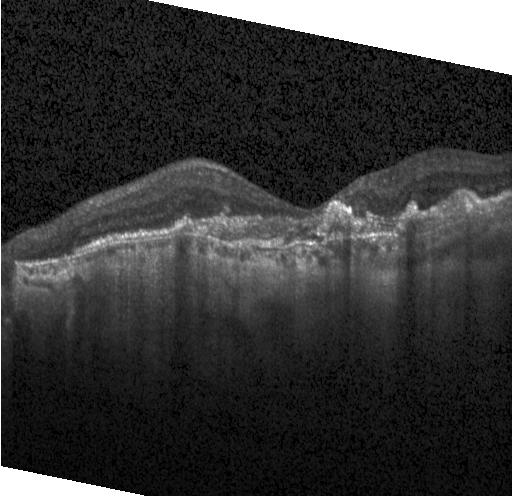 Retinal OCT cross-section; macular scan; spectral-domain optical coherence tomography.
OCT finding: CNV.